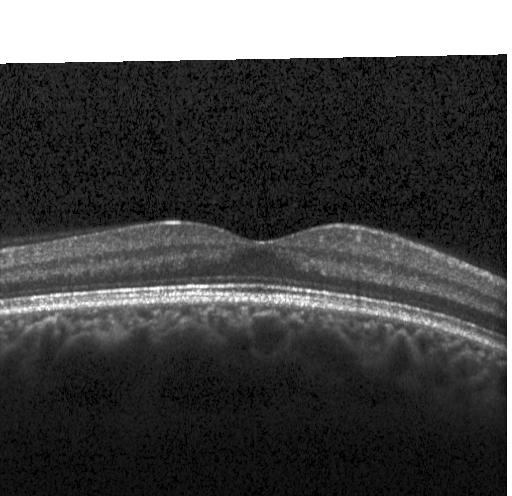
Centered on the fovea; spectral-domain OCT; instrument: Heidelberg Spectralis; optical coherence tomography scan.
This B-scan demonstrates neither choroidal neovascularization, diabetic macular edema, nor drusen.